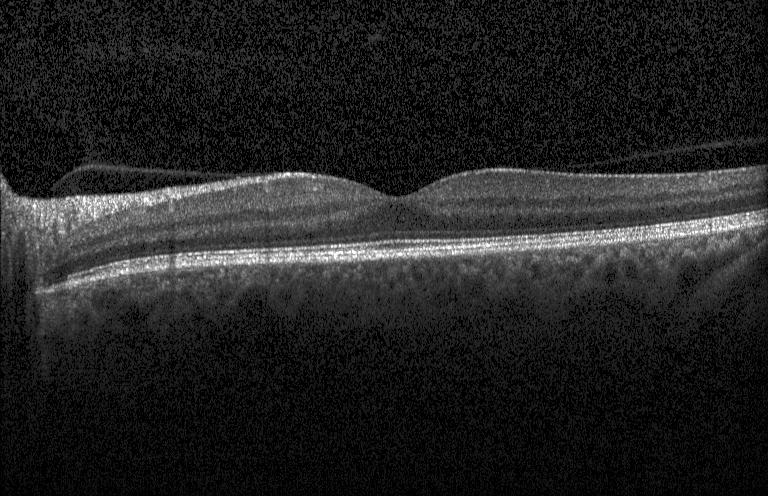
Spectral-domain optical coherence tomography · optical coherence tomography scan · Heidelberg Spectralis. Neither CNV, DME, nor drusen.